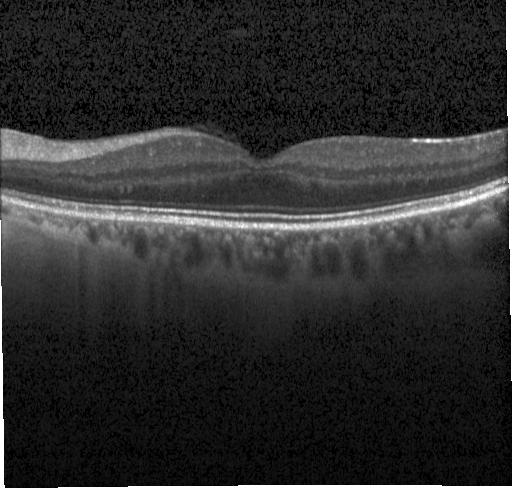 OCT B-scan showing no evidence of choroidal neovascularization, diabetic macular edema, or drusen.